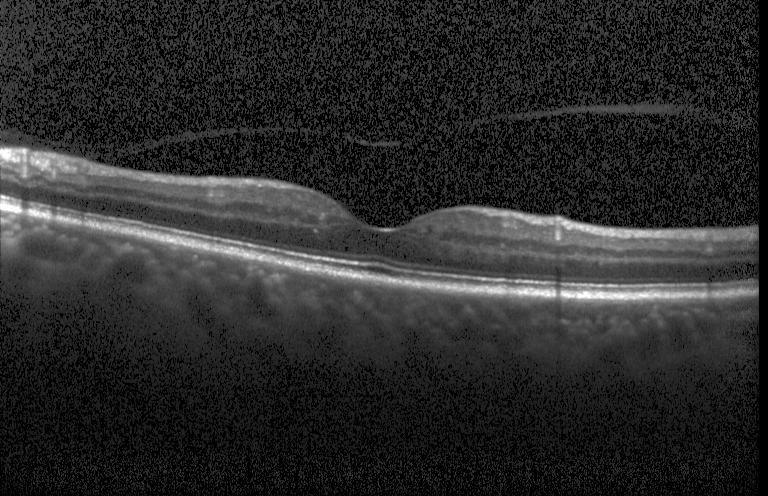
OCT line scan; SD-OCT; Heidelberg Spectralis; horizontal scan through the fovea. Macular OCT: no evidence of CNV, DME, or drusen.